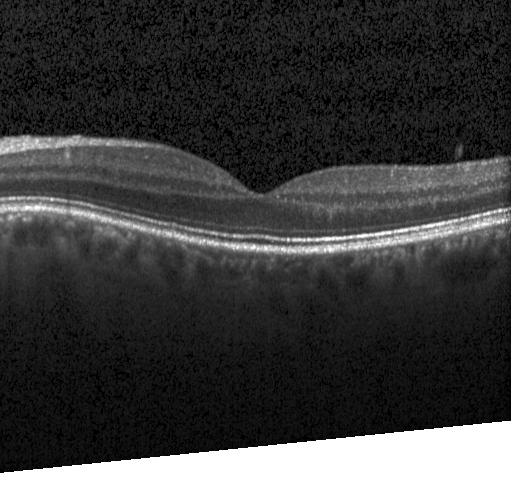

OCT B-scan · fovea-centered · spectral-domain optical coherence tomography
The scan shows no CNV, DME, or drusen.